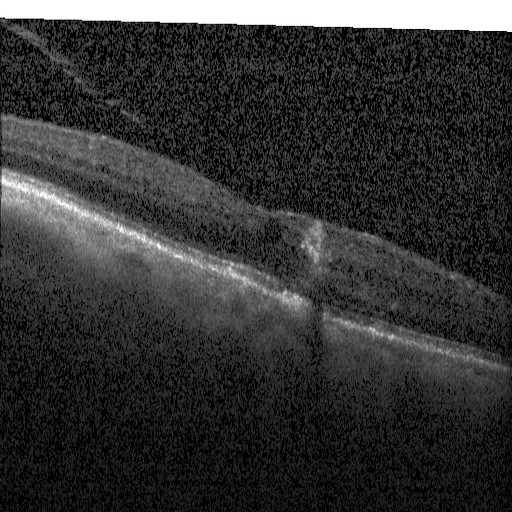

OCT B-scan
Finding: diabetic macular edema.